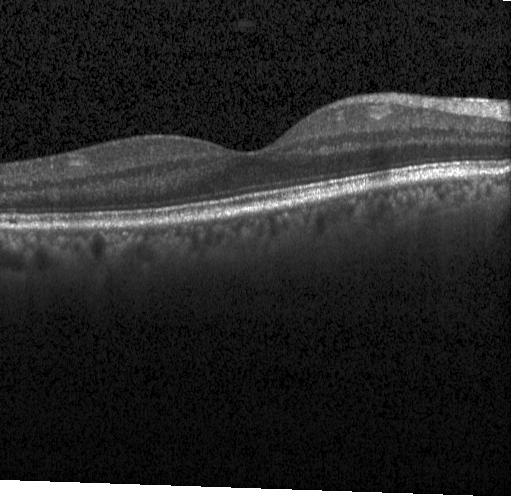
Diagnosis: no choroidal neovascularization, diabetic macular edema, or drusen.